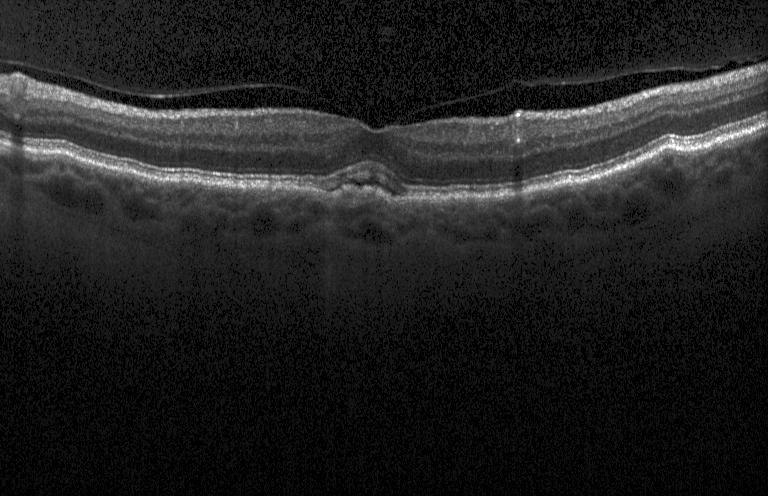
Optical coherence tomography scan, instrument: Heidelberg Spectralis. Assessment: CNV.